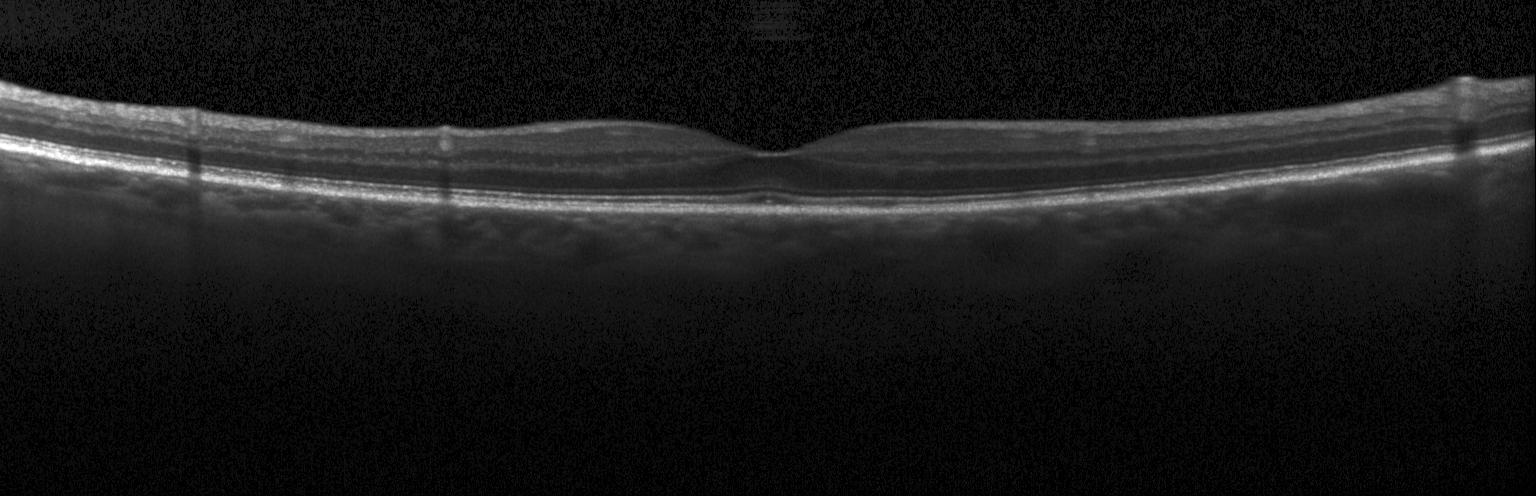
Spectral-domain OCT B-scan: no CNV, DME, or drusen.